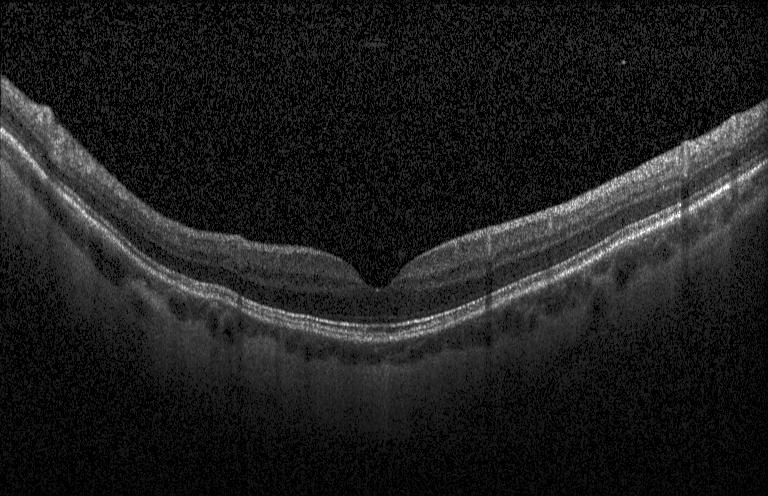

Dx: no choroidal neovascularization, no diabetic macular edema, and no drusen.